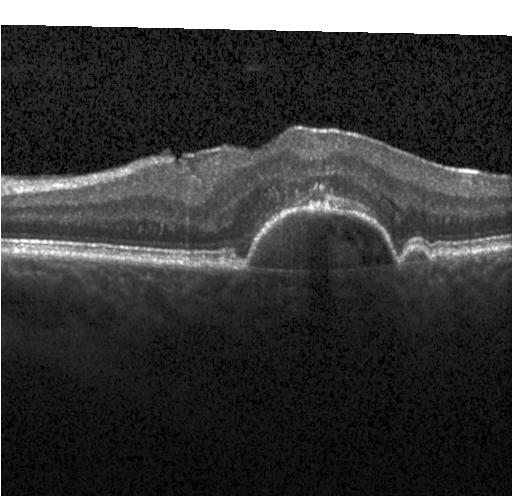

Optical coherence tomography scan · through the macula.
Impression: a choroidal neovascular membrane.